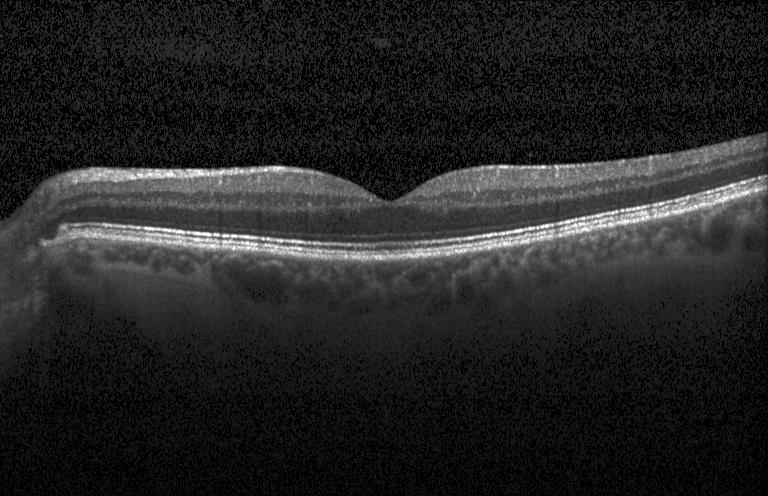 Impression: no choroidal neovascularization, diabetic macular edema, or drusen.